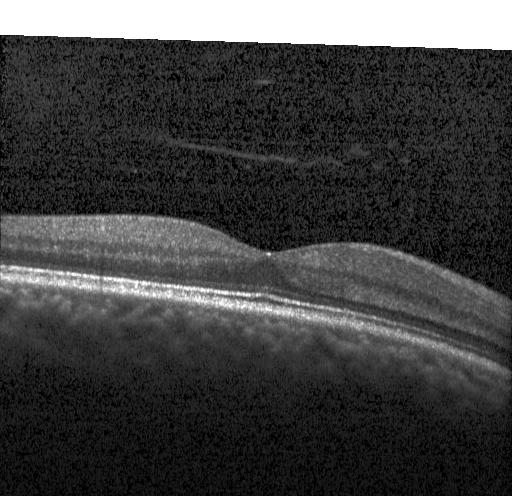
OCT line scan. Spectral-domain OCT. Diagnosis: neither choroidal neovascularization, diabetic macular edema, nor drusen.